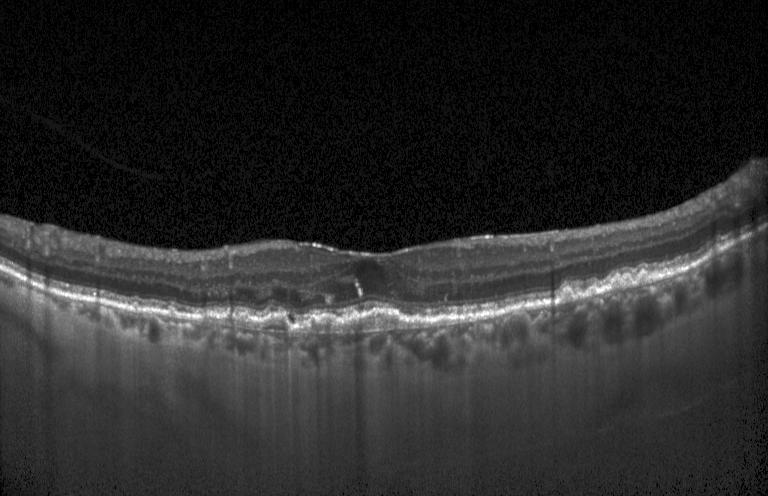

A choroidal neovascular membrane.